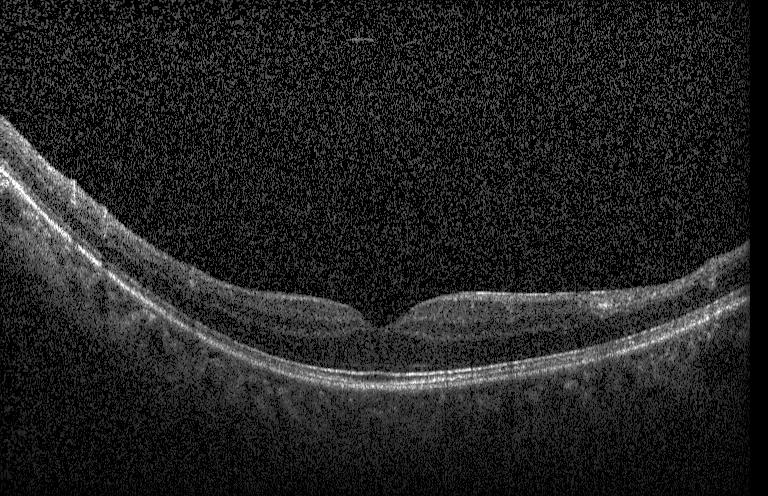 Optical coherence tomography B-scan, centered on the fovea, spectral-domain OCT. This B-scan demonstrates no evidence of choroidal neovascularization, diabetic macular edema, or drusen.